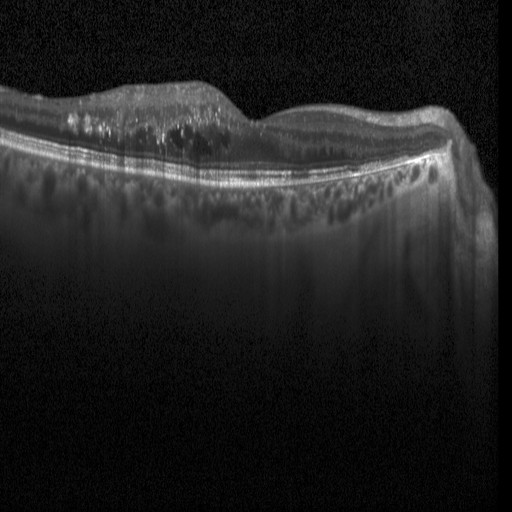

Spectral-domain OCT; optical coherence tomography scan
Diagnosis: diabetic macular edema.